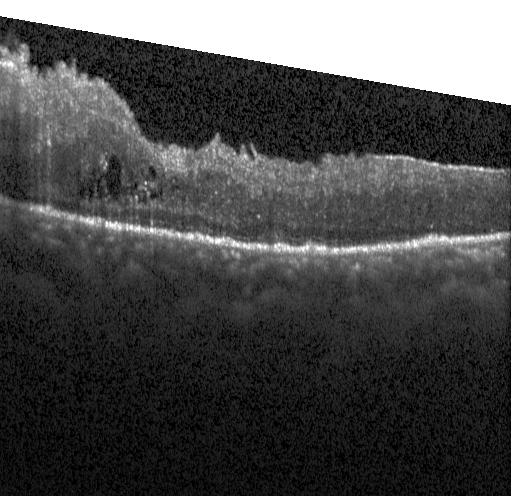 Acquired on a Heidelberg Spectralis; optical coherence tomography scan; spectral-domain OCT; horizontal scan through the fovea
Diagnosis: DME.